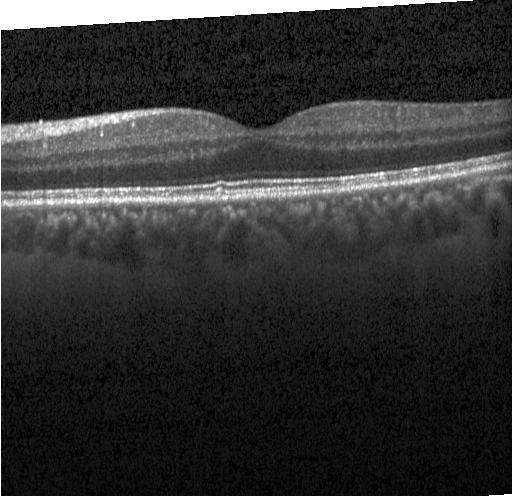
Macular scan. Retinal OCT B-scan. Spectral-domain optical coherence tomography. Heidelberg Spectralis OCT system.
OCT finding: neither choroidal neovascularization, diabetic macular edema, nor drusen.